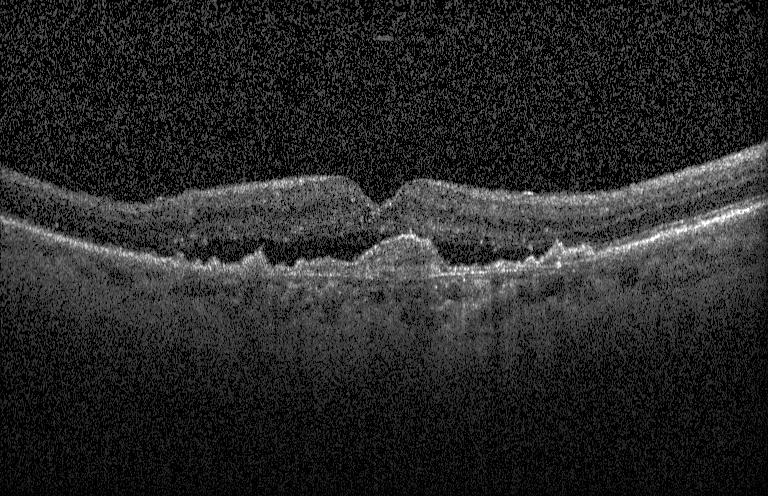 Finding: a choroidal neovascular membrane.